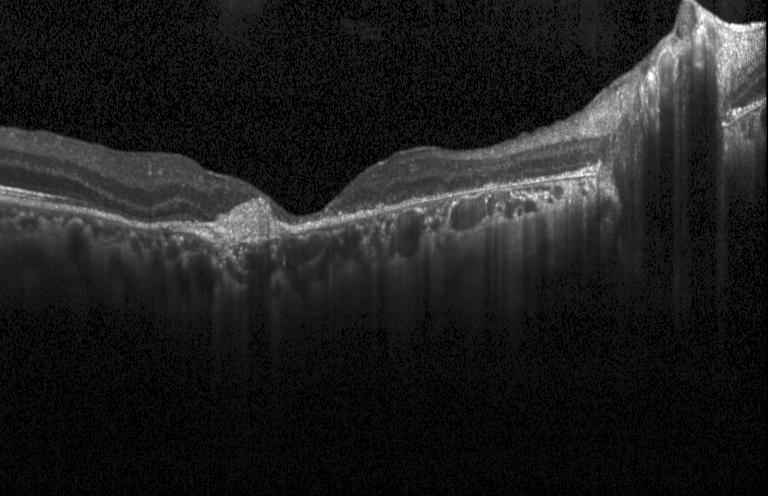 Retinal OCT B-scan.
Impression: a choroidal neovascular membrane.